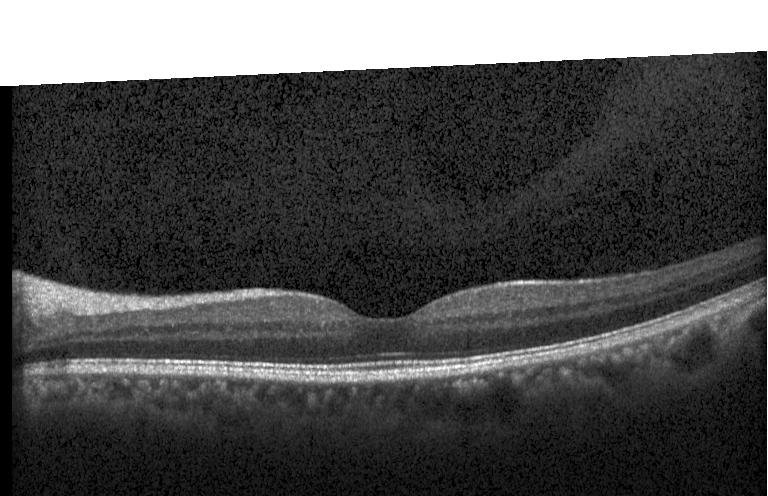

Spectral-domain optical coherence tomography, retinal OCT B-scan, instrument: Heidelberg Spectralis, macular scan — Diagnosis: no choroidal neovascularization, diabetic macular edema, or drusen.